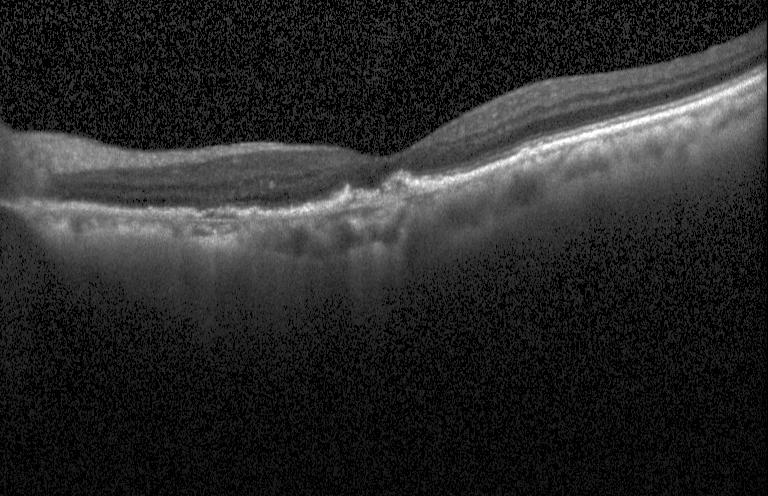
Retinal OCT B-scan.
Impression: choroidal neovascularization (CNV).